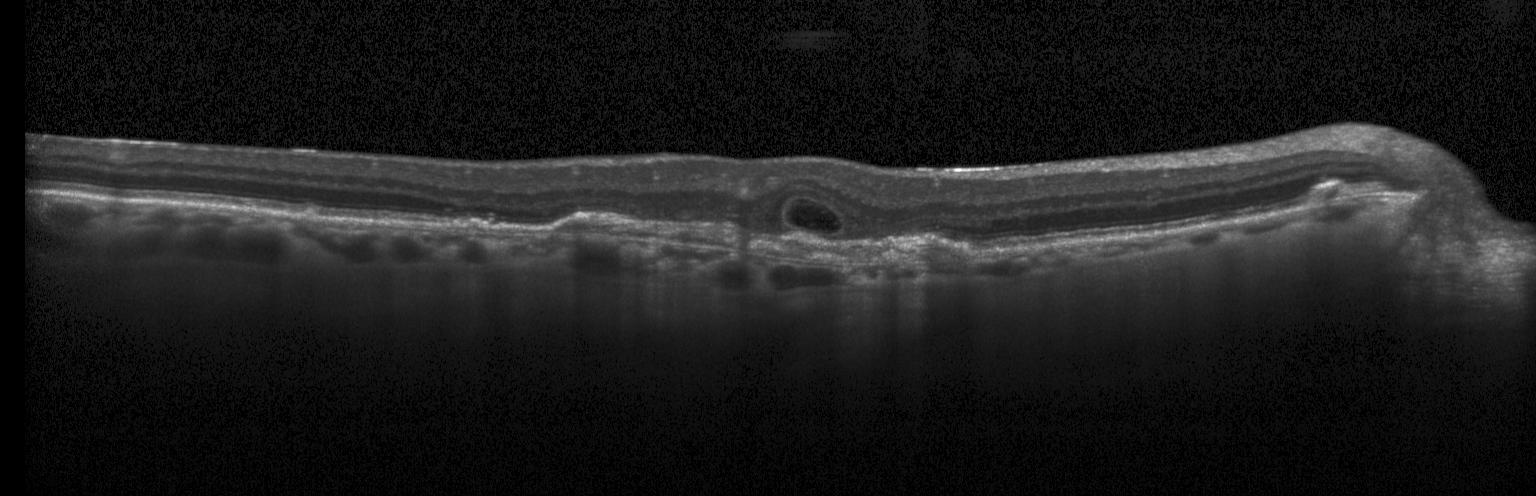
Optical coherence tomography B-scan · spectral-domain OCT · horizontal scan through the fovea · acquired on a Heidelberg Spectralis — Finding: a choroidal neovascular membrane.